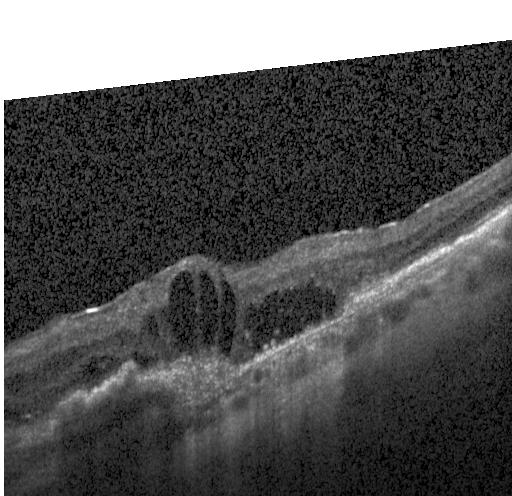 Spectral-domain OCT B-scan: a choroidal neovascular membrane.